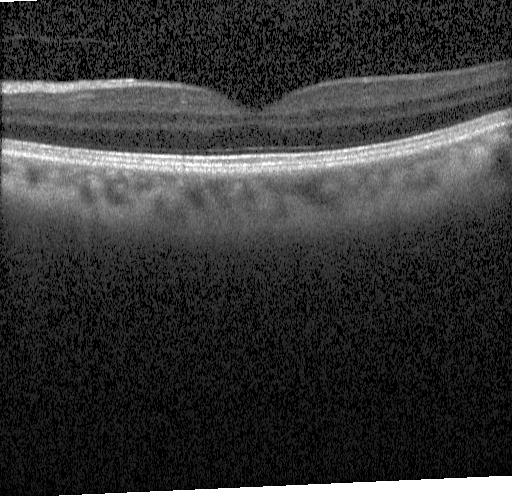 Spectral-domain optical coherence tomography; retinal OCT cross-section; through the macula — The scan shows no choroidal neovascularization, diabetic macular edema, or drusen.